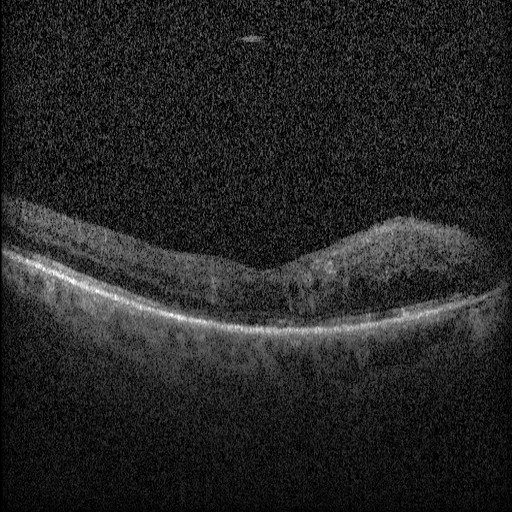
Retinal OCT cross-section showing diabetic macular edema (DME).